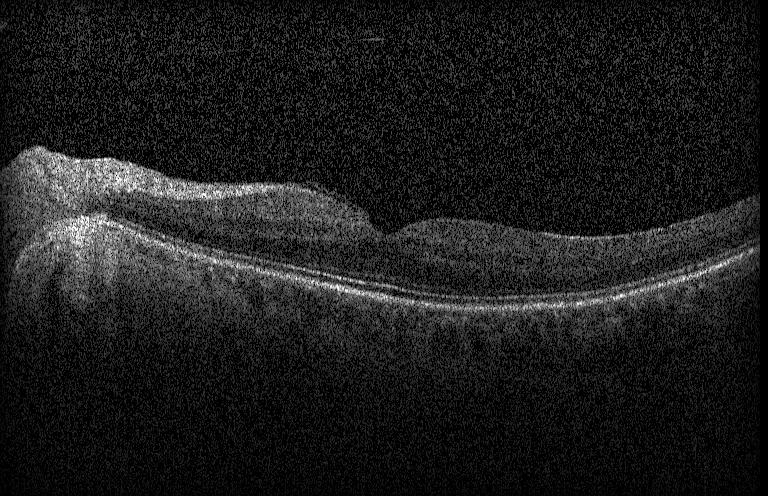
OCT finding: no choroidal neovascularization, no diabetic macular edema, and no drusen.